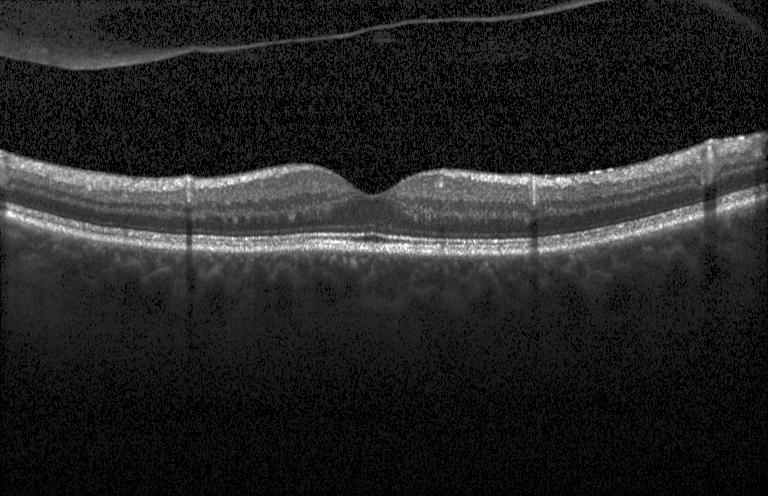

Horizontal scan through the fovea · retinal OCT cross-section — No CNV, DME, or drusen.